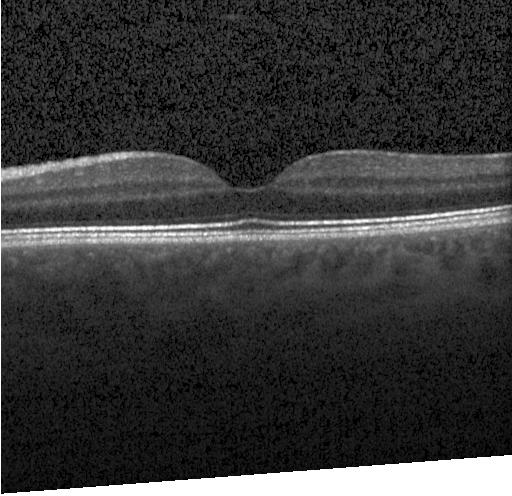
Retinal OCT cross-section, SD-OCT, Heidelberg Spectralis OCT system.
Impression: no choroidal neovascularization, no diabetic macular edema, and no drusen.